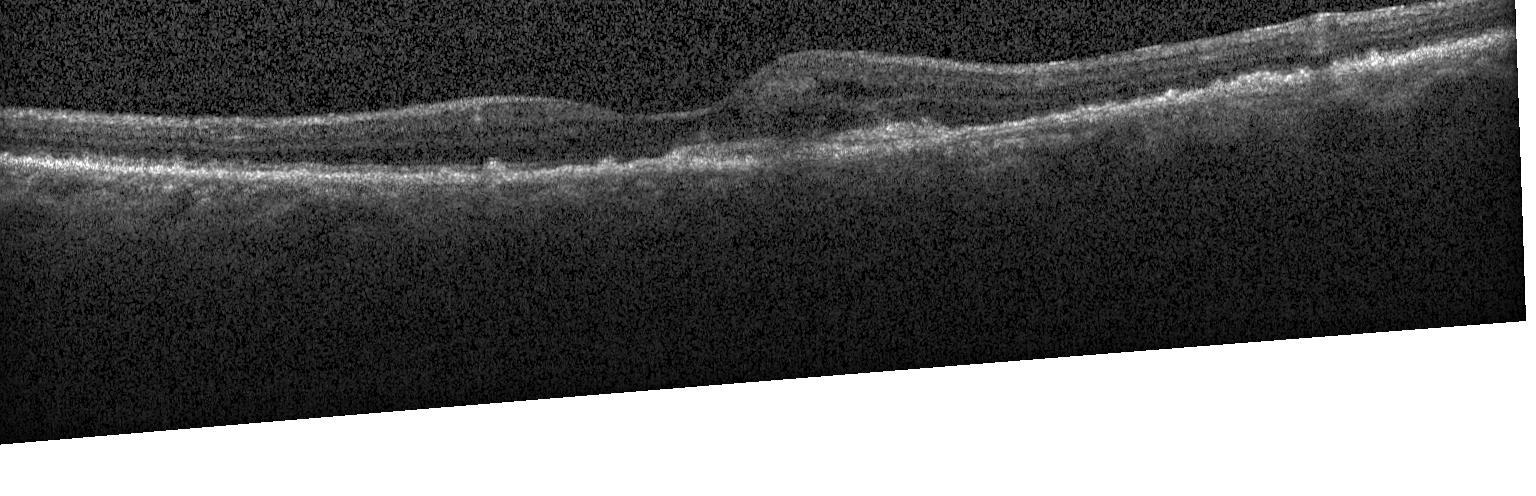 The scan shows CNV.